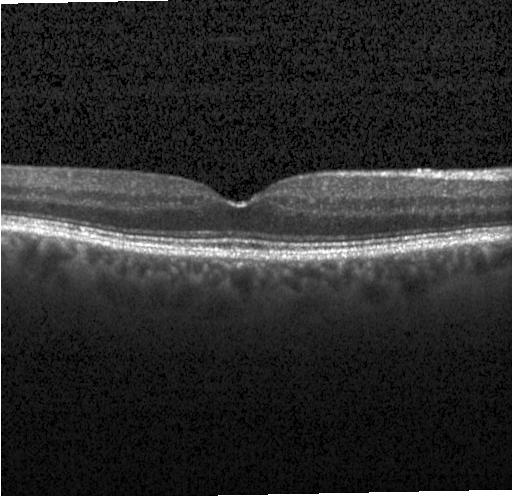

Optical coherence tomography B-scan, Heidelberg Spectralis, macular scan. No choroidal neovascularization, diabetic macular edema, or drusen.